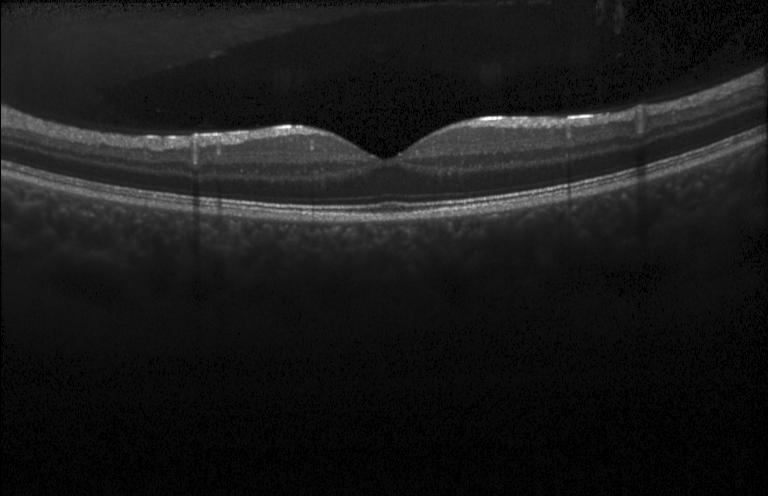

SD-OCT. OCT line scan. Horizontal scan through the fovea. Dx: no choroidal neovascularization, diabetic macular edema, or drusen.